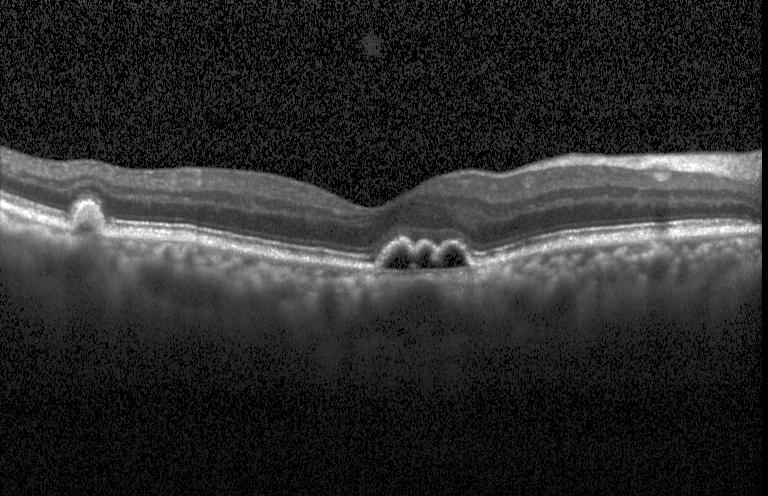

OCT B-scan, instrument: Heidelberg Spectralis, fovea-centered — OCT finding: a choroidal neovascular membrane.